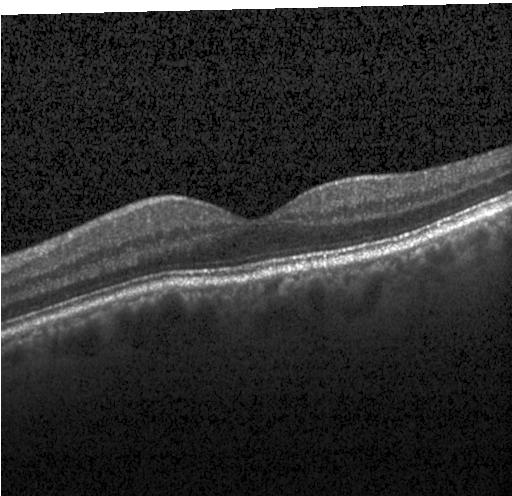

Spectral-domain OCT B-scan: no evidence of CNV, DME, or drusen.